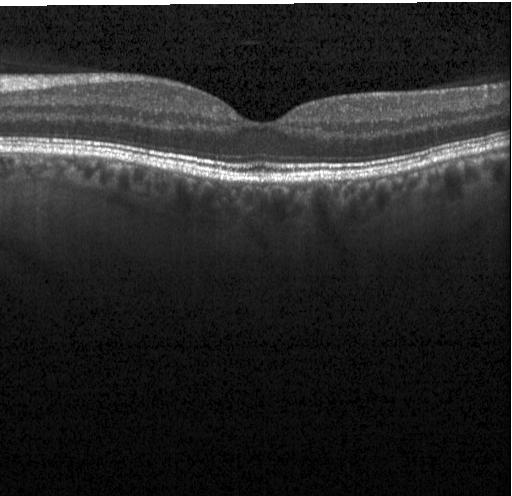 Fovea-centered. OCT line scan. Spectral-domain optical coherence tomography. Finding: no evidence of choroidal neovascularization, diabetic macular edema, or drusen.